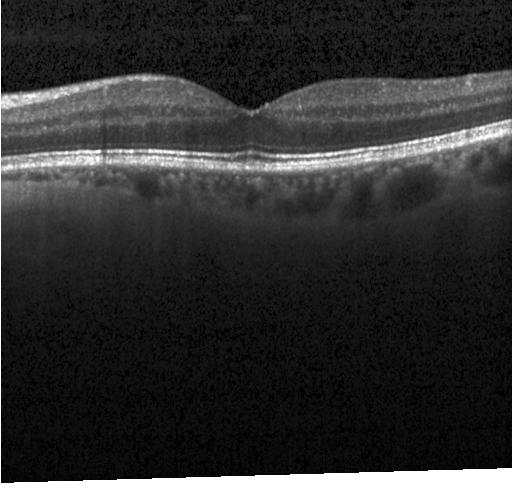 Retinal OCT cross-section.
Diagnosis: neither choroidal neovascularization, diabetic macular edema, nor drusen.